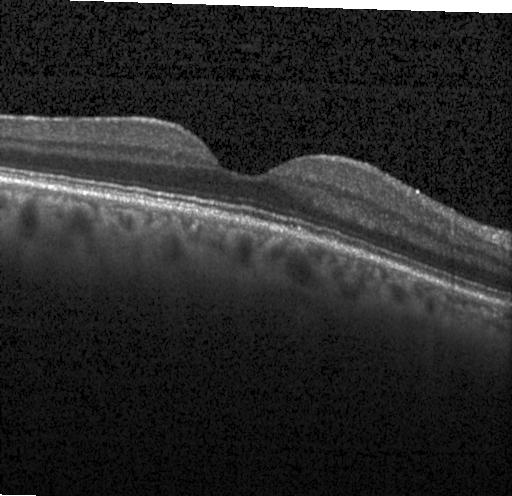
OCT line scan — The scan shows no evidence of choroidal neovascularization, diabetic macular edema, or drusen.